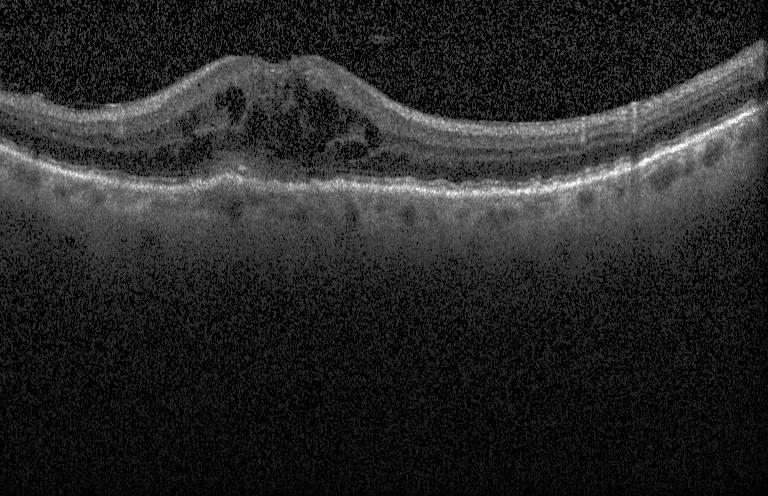
Spectral-domain optical coherence tomography. Through the macula. Retinal OCT cross-section
Assessment: a choroidal neovascular membrane.